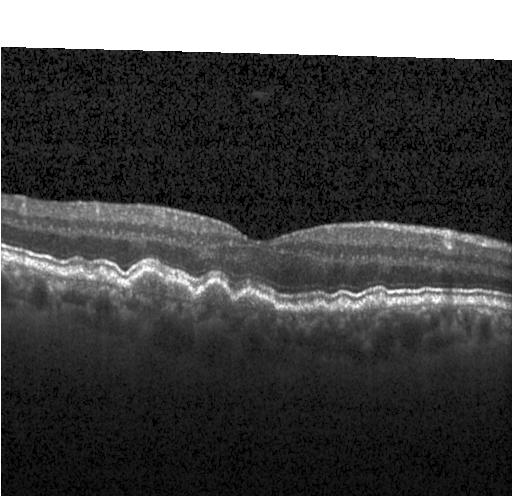
Impression: multiple drusen.